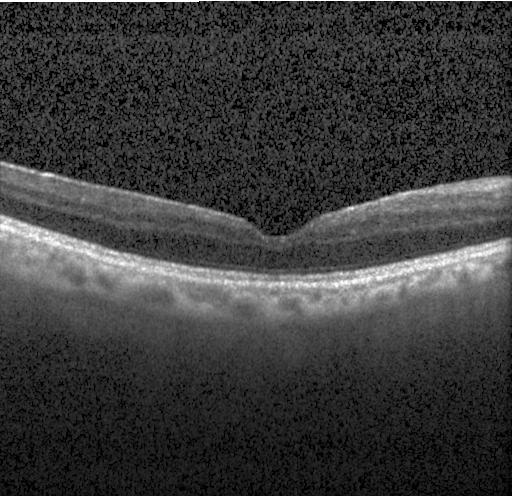 OCT finding: no choroidal neovascularization, diabetic macular edema, or drusen.